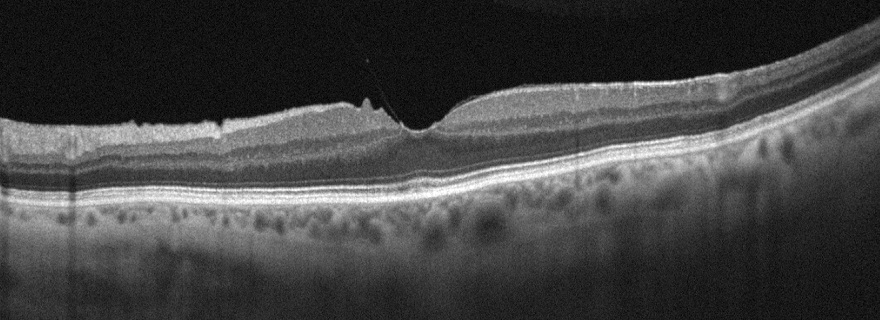
Epiretinal membrane (ERM).